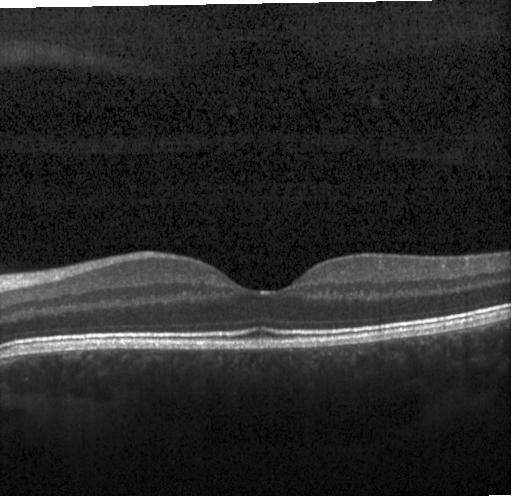
Through the macula. Acquired on a Heidelberg Spectralis. Spectral-domain optical coherence tomography. OCT B-scan. Diagnosis: neither choroidal neovascularization, diabetic macular edema, nor drusen.